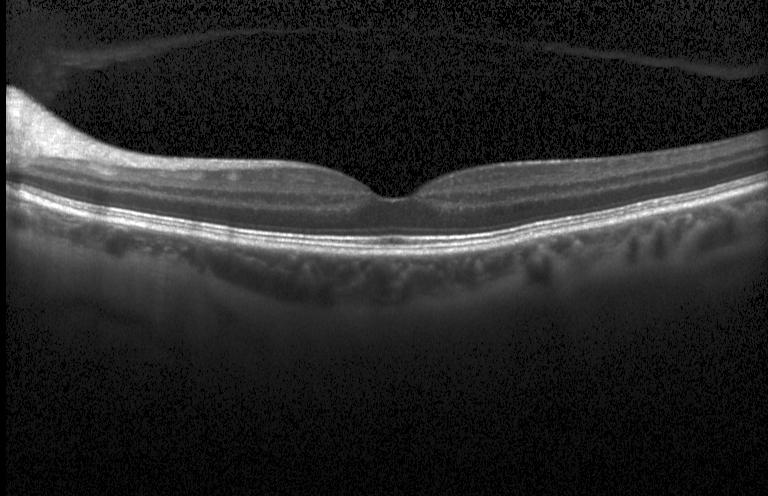
Optical coherence tomography B-scan, spectral-domain OCT.
Diagnosis: no choroidal neovascularization, no diabetic macular edema, and no drusen.